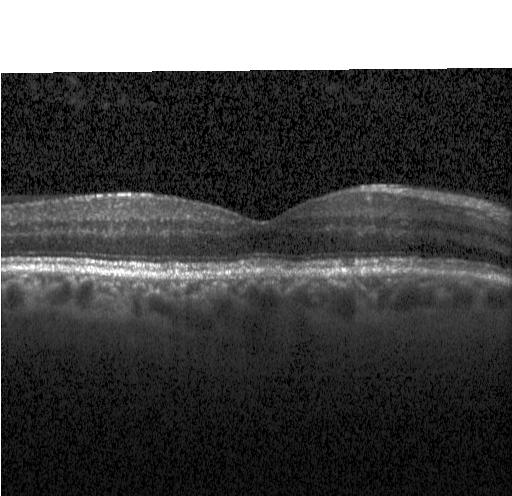 Impression: no choroidal neovascularization, diabetic macular edema, or drusen.